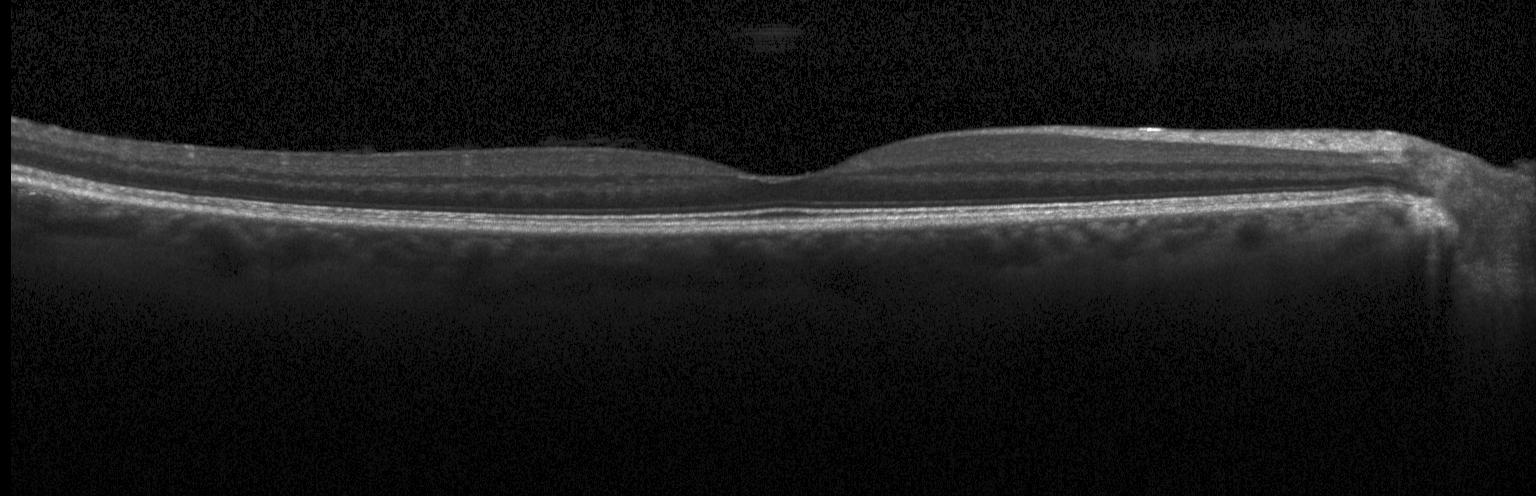
Through the macula · OCT line scan · SD-OCT.
The scan shows no evidence of CNV, DME, or drusen.